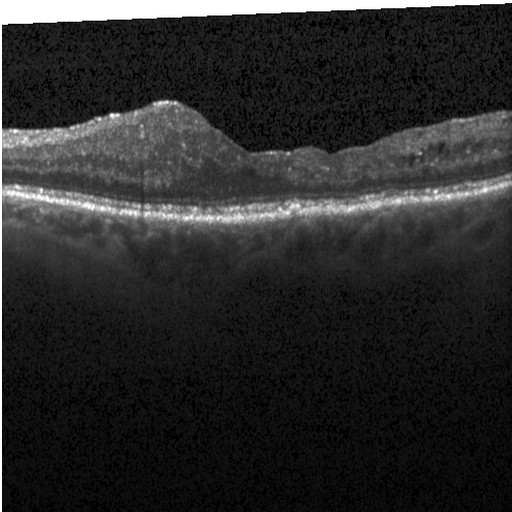 Diagnosis: diabetic macular edema (DME).